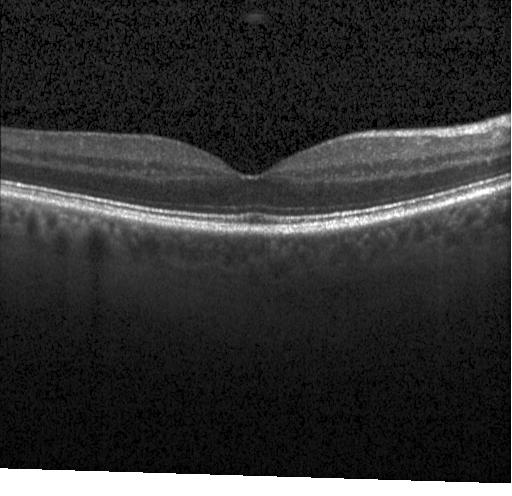 Finding: no choroidal neovascularization, diabetic macular edema, or drusen.